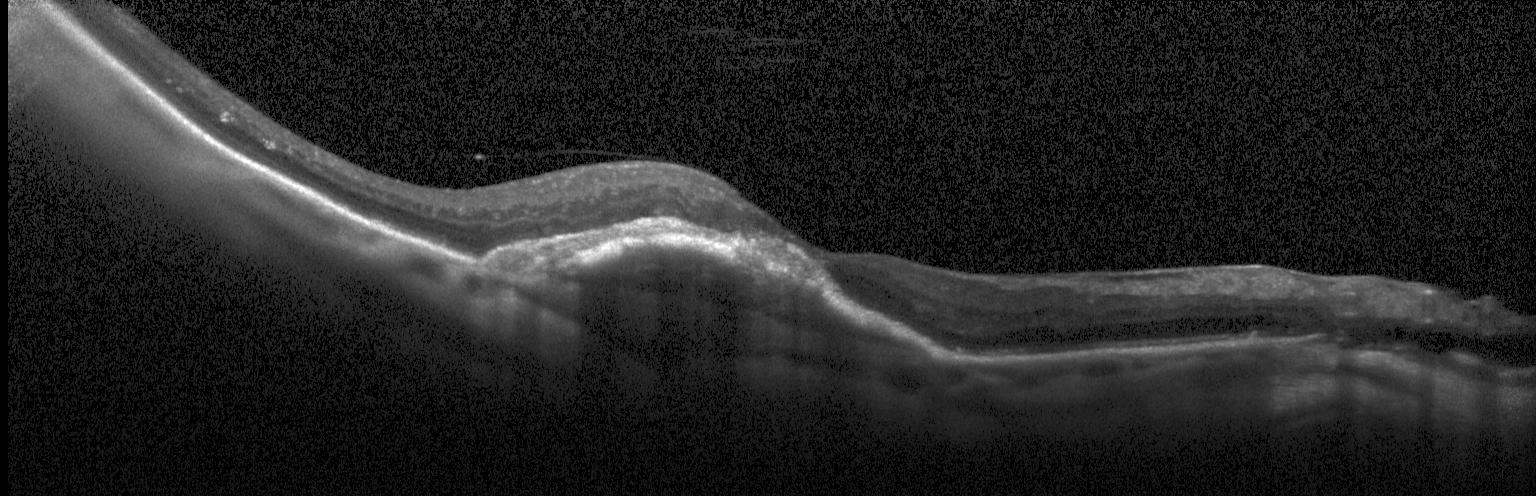
Diagnosis: choroidal neovascularization (CNV).